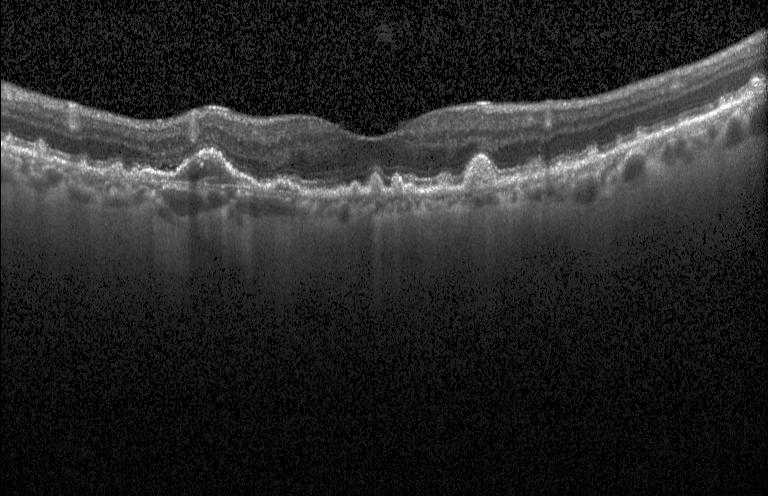

Horizontal scan through the fovea, optical coherence tomography scan, Heidelberg Spectralis OCT system. Diagnosis: sub-RPE drusenoid deposits.